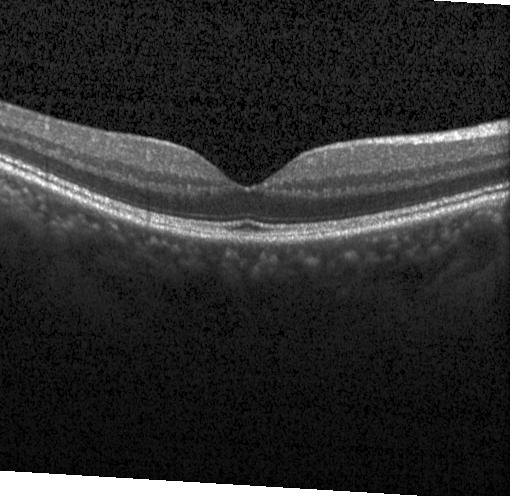 Retinal OCT B-scan. Macular OCT: neither CNV, DME, nor drusen.